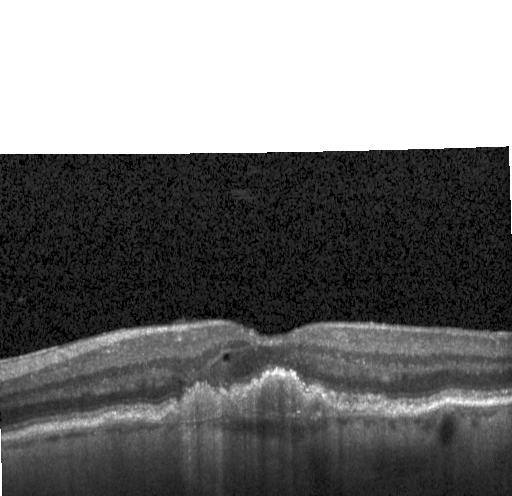 Through the macula, instrument: Heidelberg Spectralis, retinal OCT B-scan. Impression: a choroidal neovascular membrane.